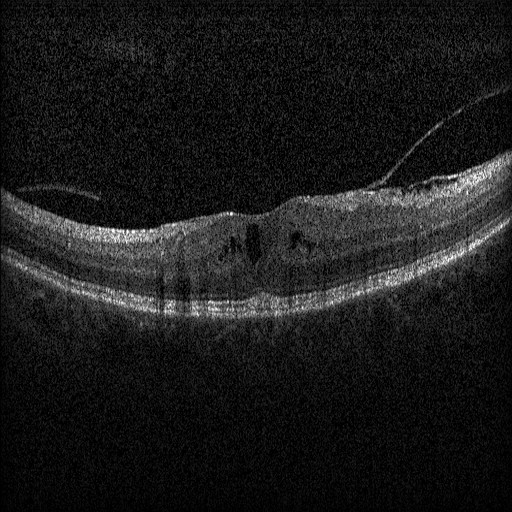

Retinal OCT cross-section, horizontal scan through the fovea, SD-OCT, Heidelberg Spectralis — Impression: diabetic macular edema (DME).